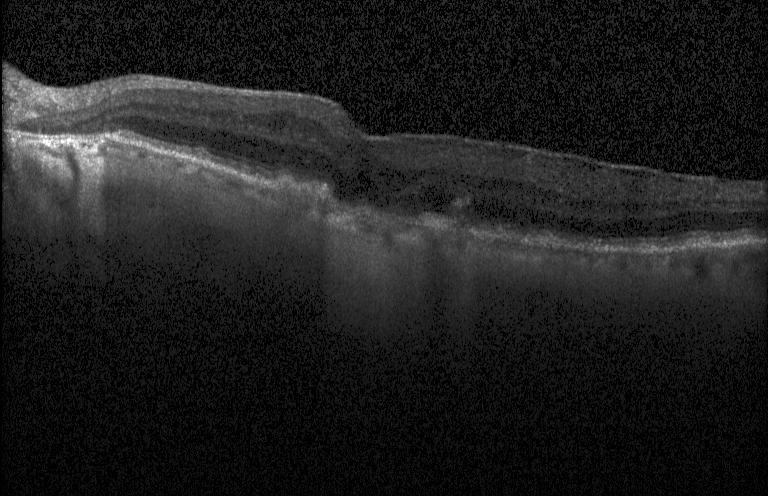
Retinal OCT cross-section — Diagnosis: a choroidal neovascular membrane.